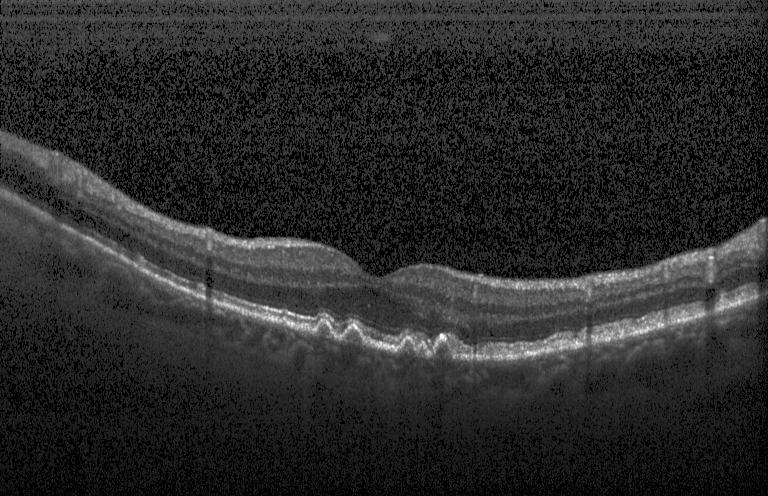

Dx: sub-RPE drusenoid deposits.